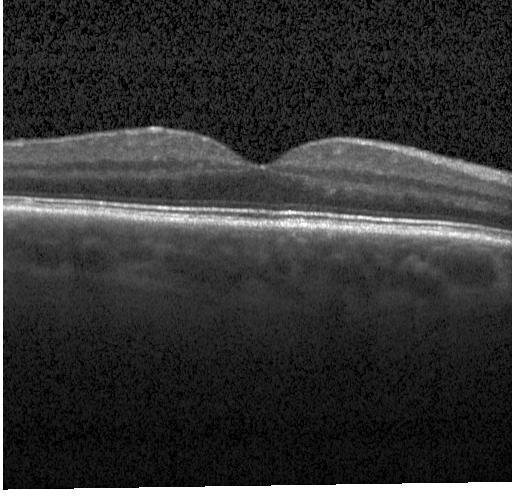 No CNV, no DME, and no drusen.